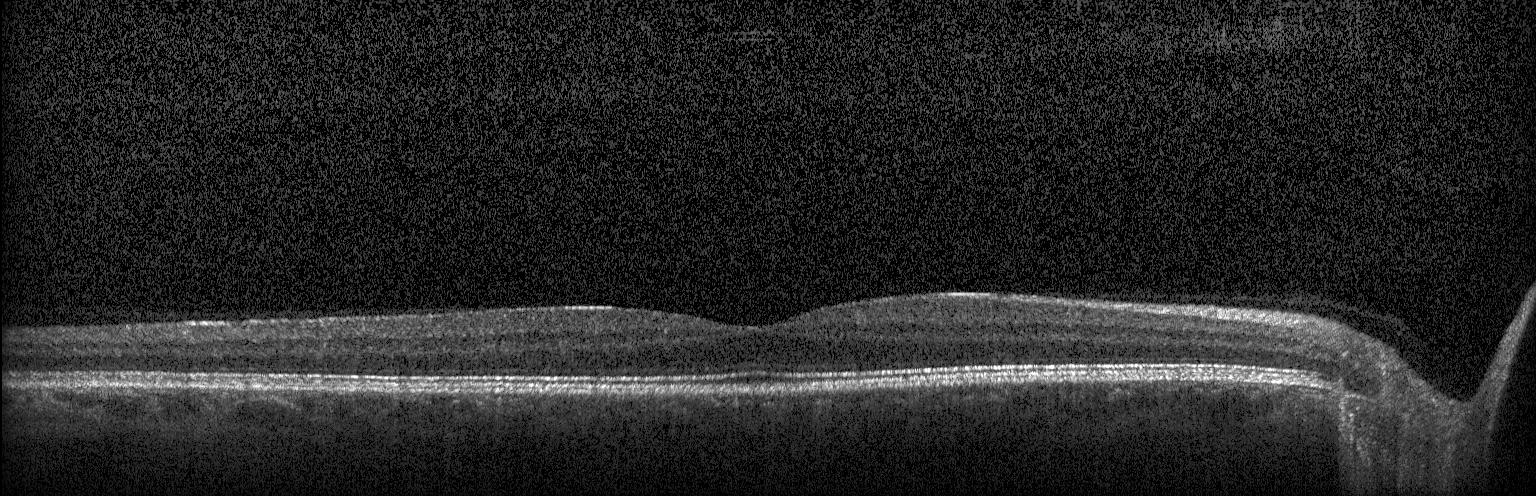
Diagnosis: no choroidal neovascularization, diabetic macular edema, or drusen.